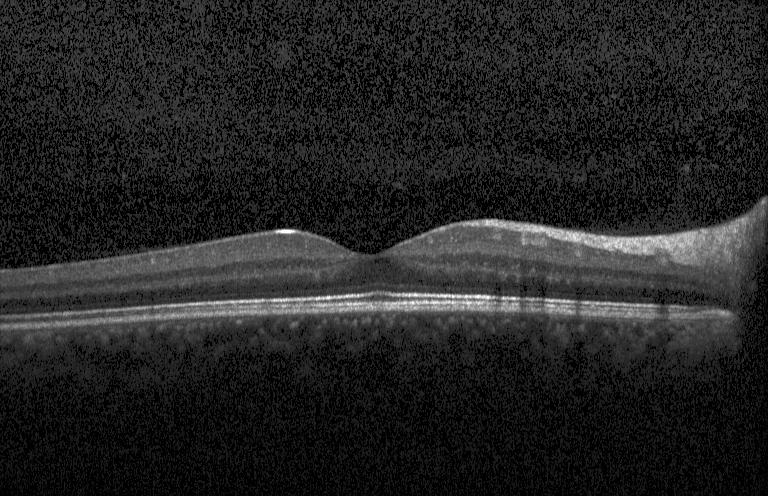 Retinal OCT cross-section — Diagnosis: no choroidal neovascularization, no diabetic macular edema, and no drusen.